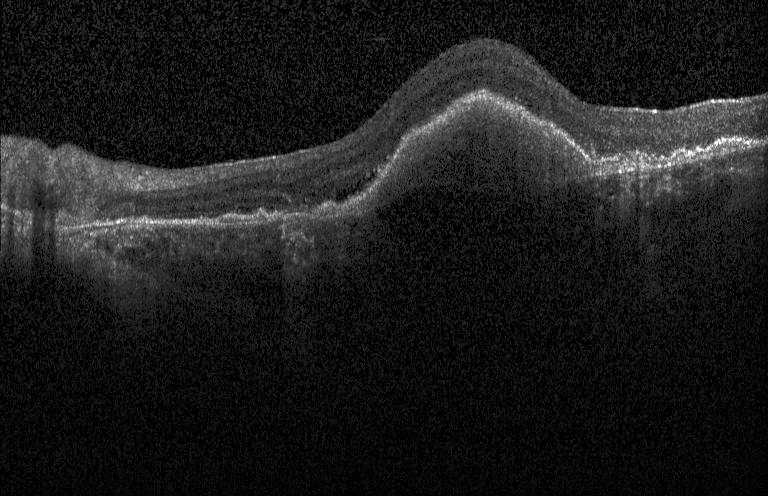

Acquired on a Heidelberg Spectralis. Retinal OCT B-scan. Spectral-domain optical coherence tomography.
Diagnosis: choroidal neovascularization.